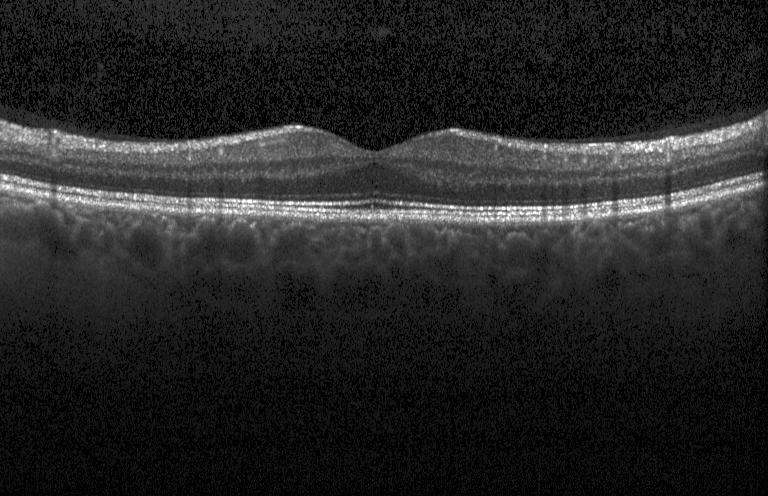 Acquired on a Heidelberg Spectralis. Optical coherence tomography B-scan — Impression: no evidence of CNV, DME, or drusen.